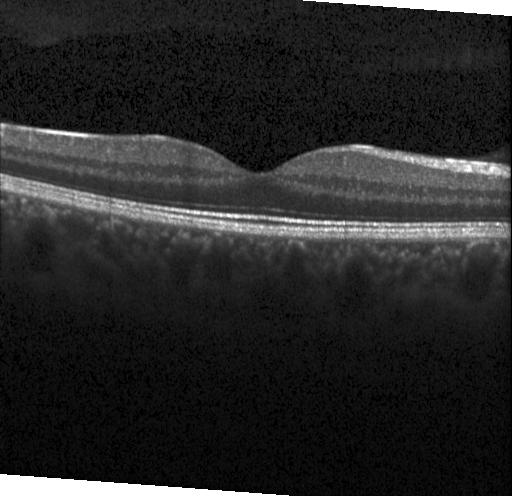

Diagnosis: neither choroidal neovascularization, diabetic macular edema, nor drusen.